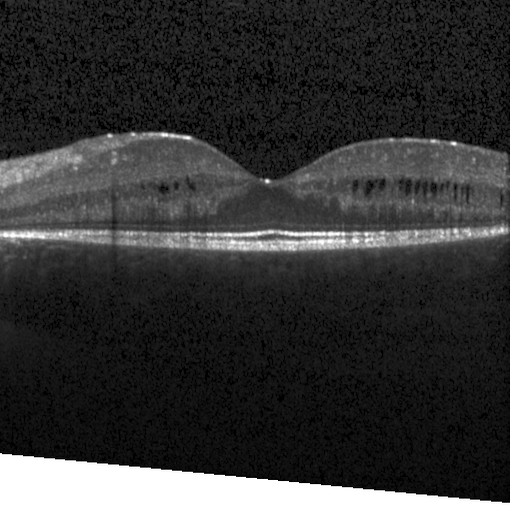

Retinal OCT cross-section.
Impression: diabetic macular edema (DME).